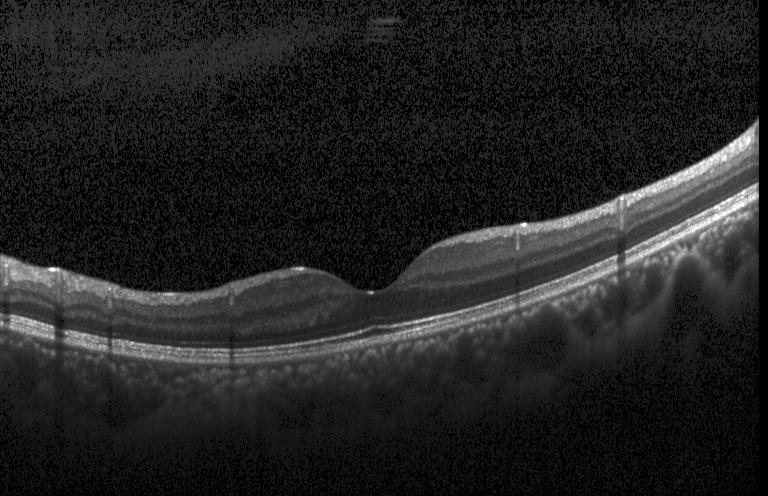

Optical coherence tomography scan · through the macula · spectral-domain OCT · Heidelberg Spectralis OCT system.
Assessment: neither choroidal neovascularization, diabetic macular edema, nor drusen.